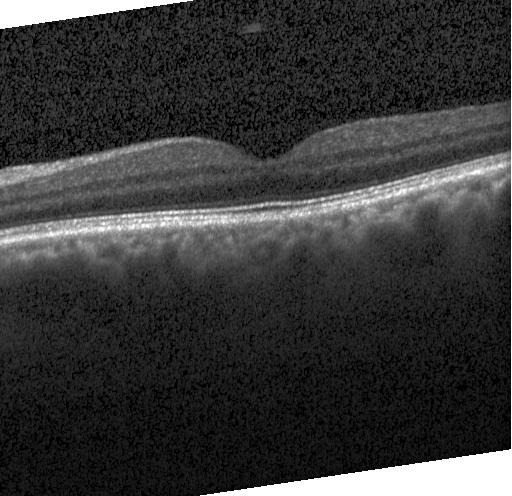 Diagnosis: no CNV, DME, or drusen.